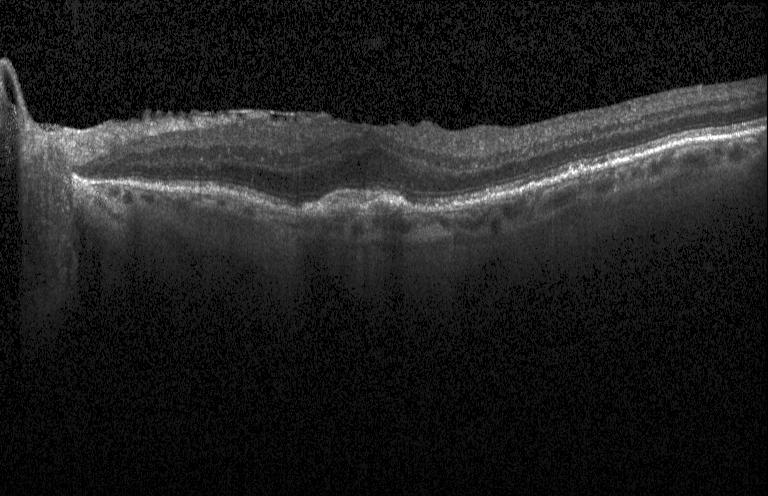
OCT B-scan. Acquired on a Heidelberg Spectralis — OCT finding: a choroidal neovascular membrane.